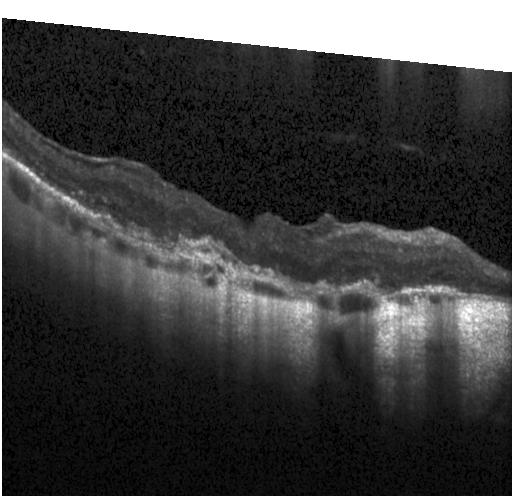
Spectral-domain optical coherence tomography · through the macula · OCT B-scan — OCT finding: choroidal neovascularization (CNV).